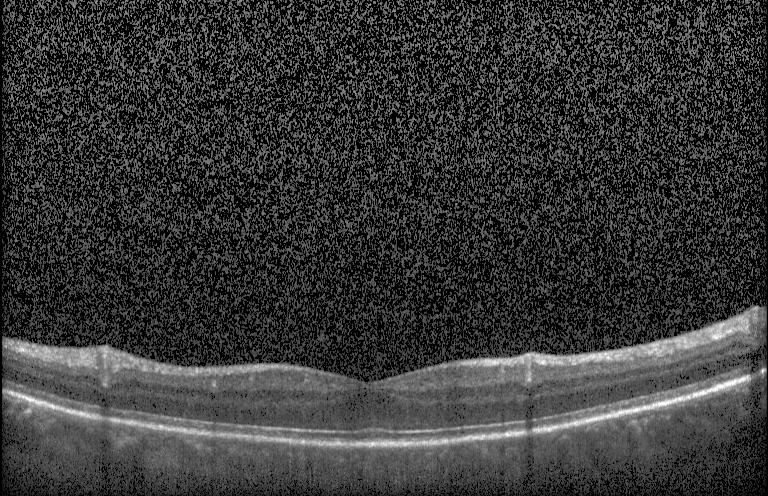

Acquired on a Heidelberg Spectralis. Horizontal scan through the fovea. Retinal OCT B-scan
Neither choroidal neovascularization, diabetic macular edema, nor drusen.